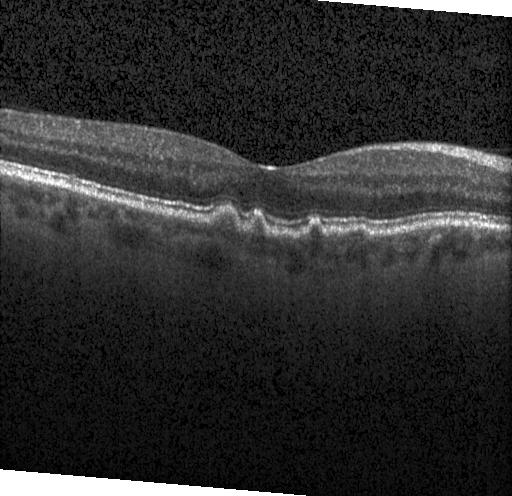 Retinal OCT cross-section; spectral-domain optical coherence tomography — Assessment: drusen.